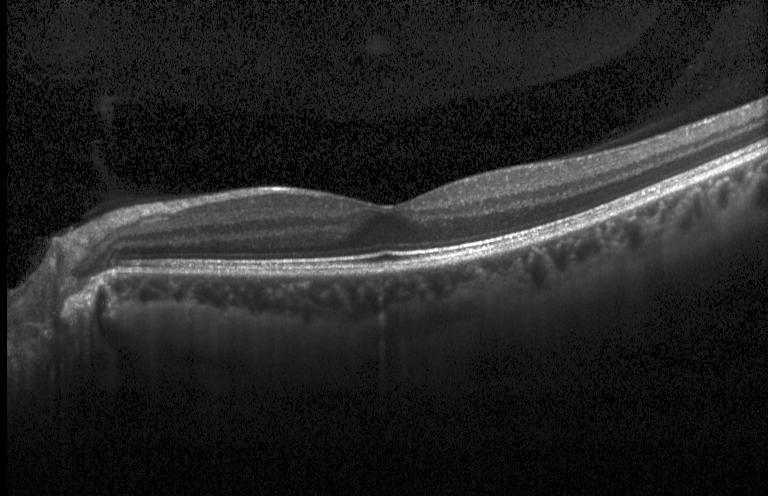

OCT finding: no CNV, DME, or drusen.